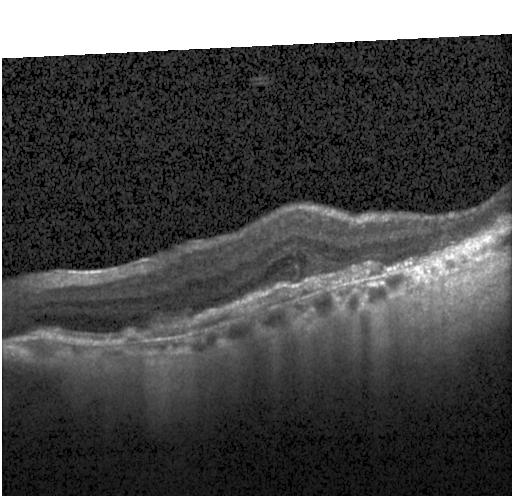

Assessment: a choroidal neovascular membrane.